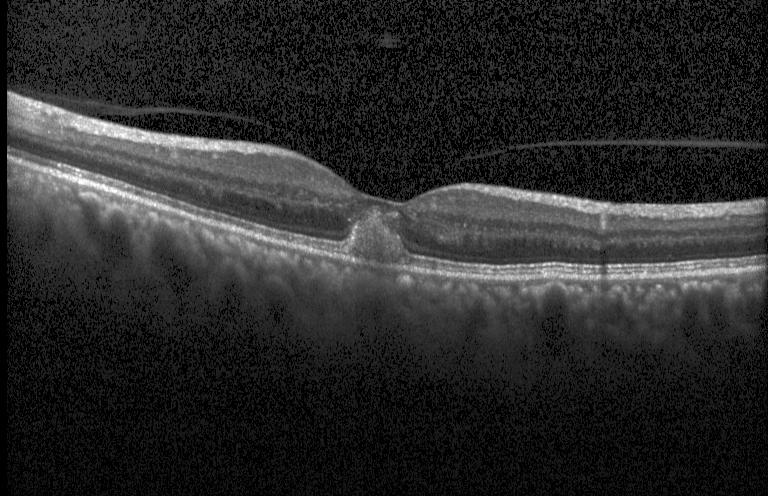 Retinal OCT B-scan. Heidelberg Spectralis OCT system. Macular OCT: a choroidal neovascular membrane.